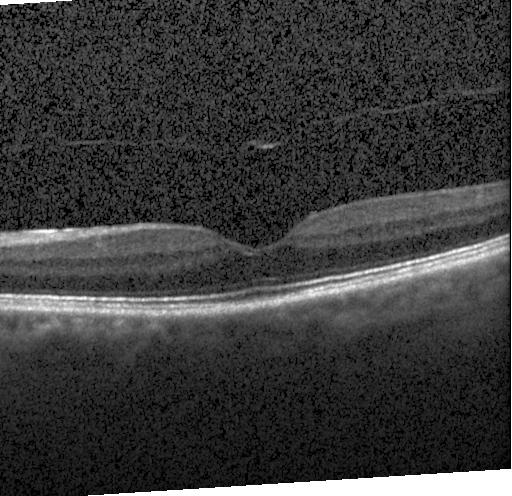 Retinal OCT cross-section.
Assessment: no CNV, no DME, and no drusen.